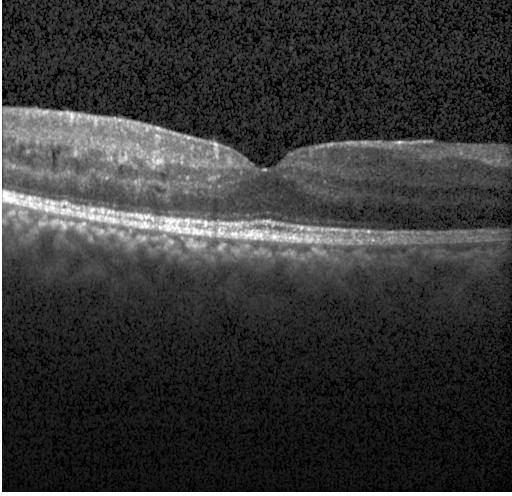 The scan shows diabetic macular edema.